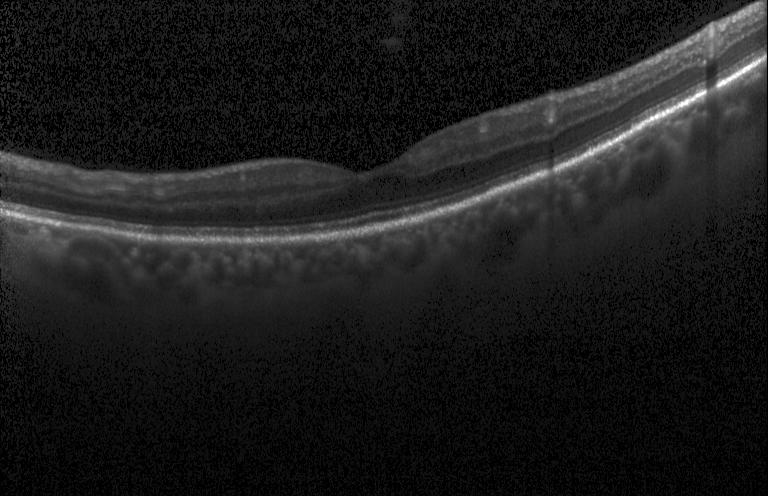

Macular OCT: neither choroidal neovascularization, diabetic macular edema, nor drusen.